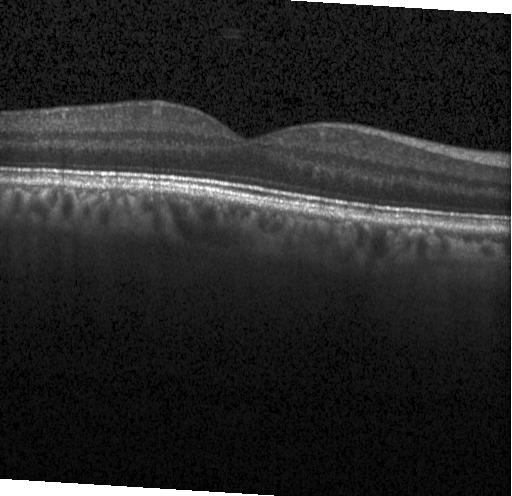 Centered on the fovea. Optical coherence tomography scan. Heidelberg Spectralis — Diagnosis: neither choroidal neovascularization, diabetic macular edema, nor drusen.